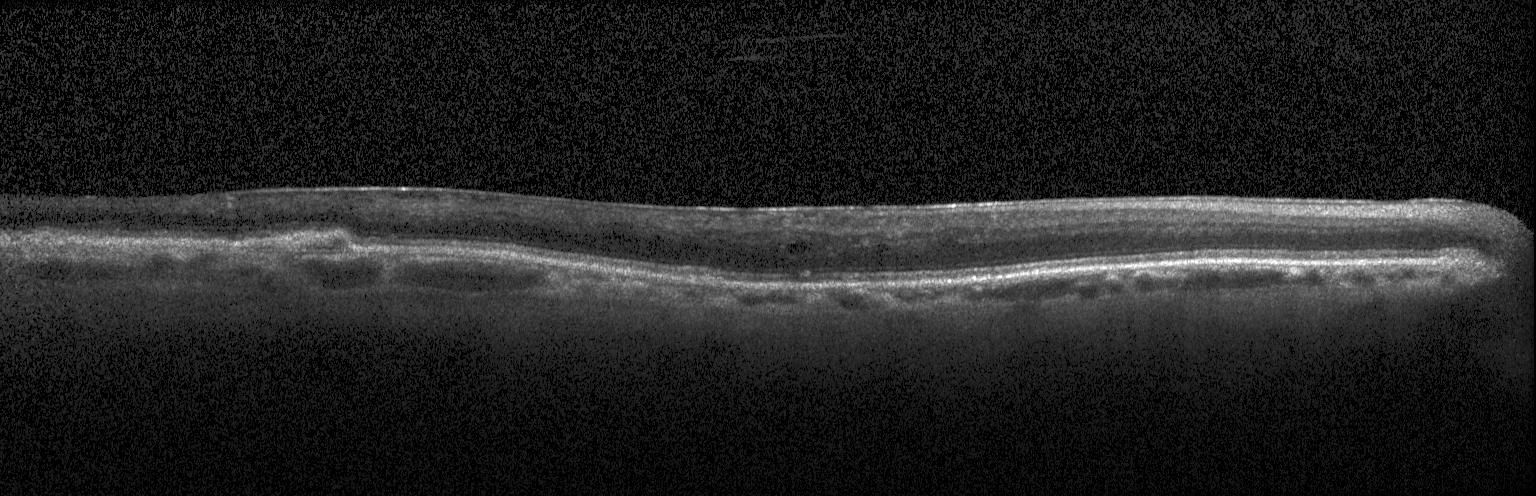 OCT line scan. Macular OCT: CNV.